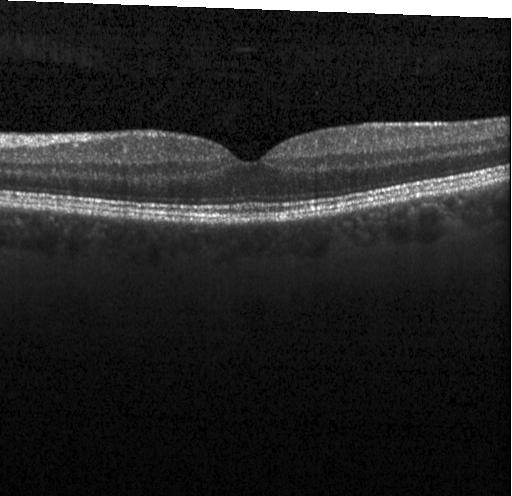
Optical coherence tomography scan — Finding: neither CNV, DME, nor drusen.